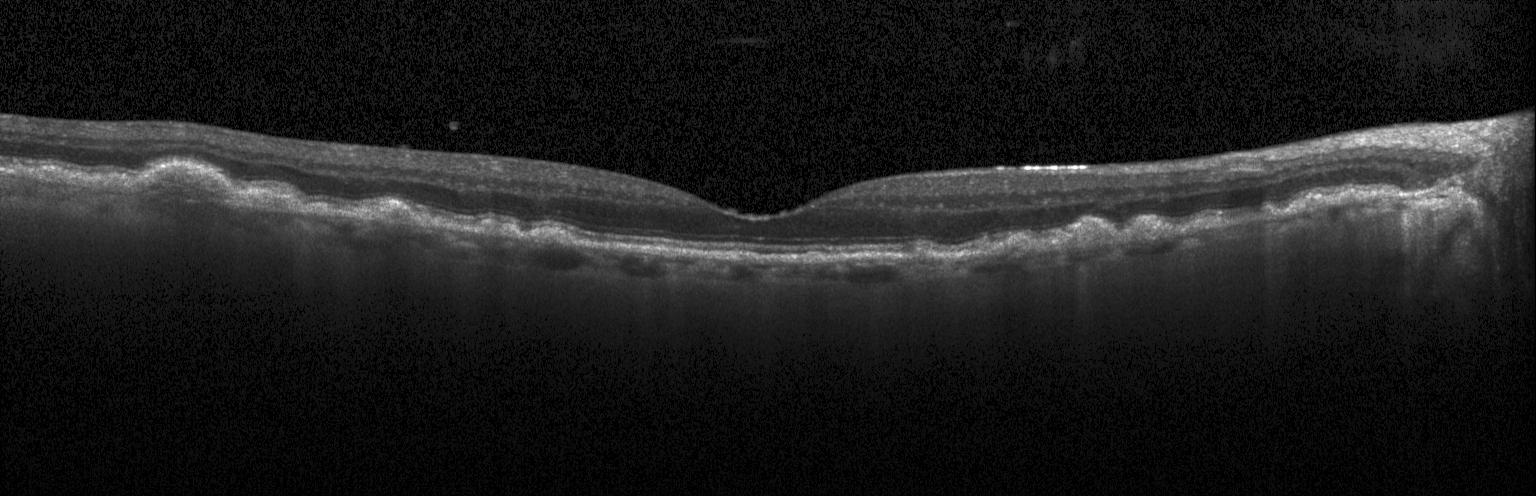
The scan shows drusen.